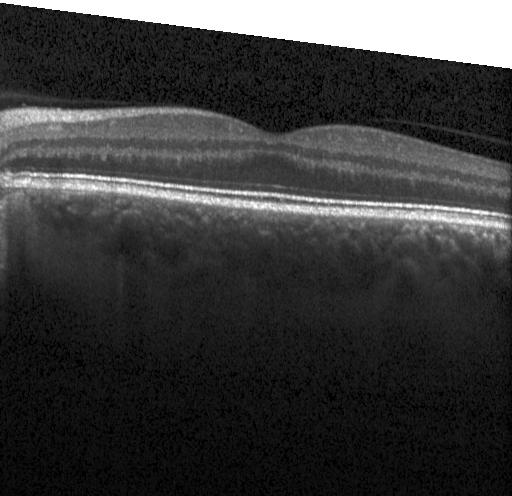
Retinal OCT cross-section.
OCT finding: neither choroidal neovascularization, diabetic macular edema, nor drusen.